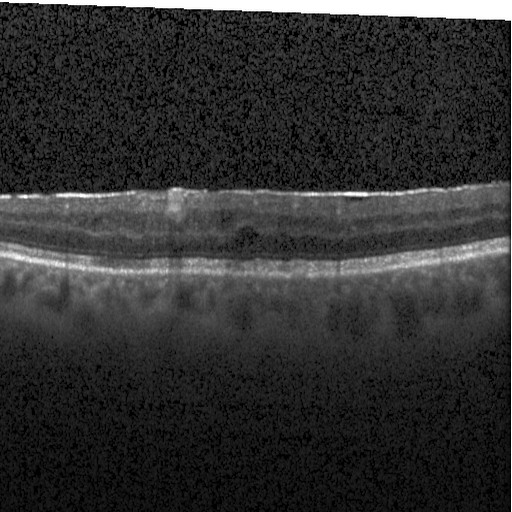

Optical coherence tomography B-scan, centered on the fovea.
Dx: diabetic macular edema (DME).